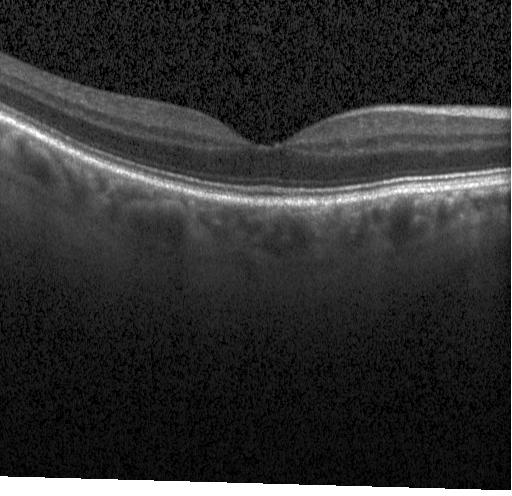 Spectral-domain OCT; instrument: Heidelberg Spectralis; through the macula; retinal OCT cross-section — No choroidal neovascularization, diabetic macular edema, or drusen.